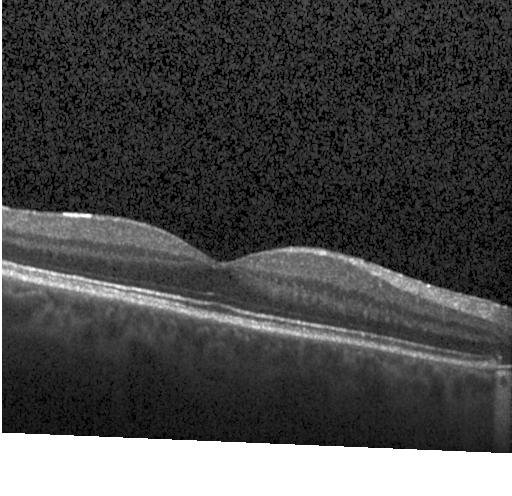 OCT B-scan · fovea-centered · Heidelberg Spectralis OCT system — Diagnosis: no evidence of choroidal neovascularization, diabetic macular edema, or drusen.